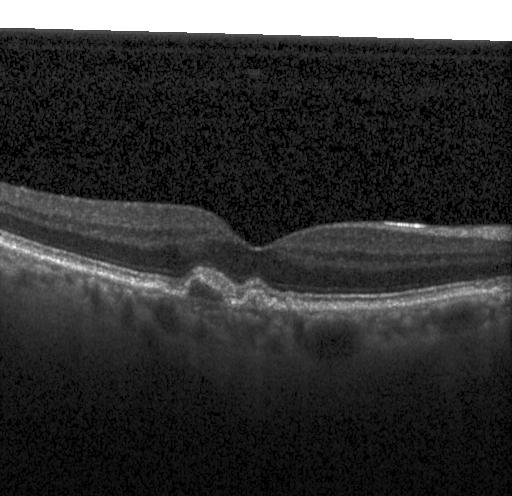

Retinal OCT B-scan; SD-OCT; through the macula; Heidelberg Spectralis OCT system. Impression: CNV.